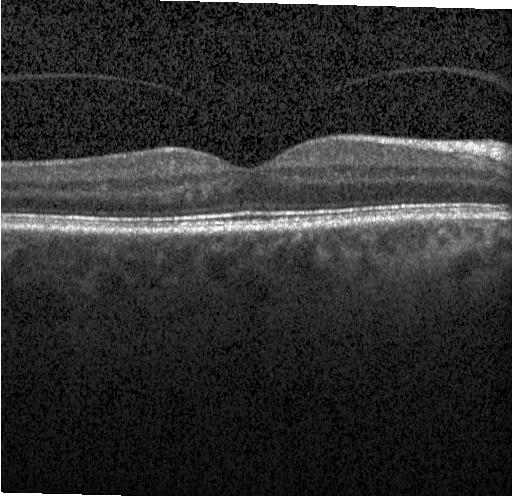
Through the macula. Spectral-domain optical coherence tomography. Heidelberg Spectralis. Retinal OCT B-scan. This B-scan demonstrates neither CNV, DME, nor drusen.